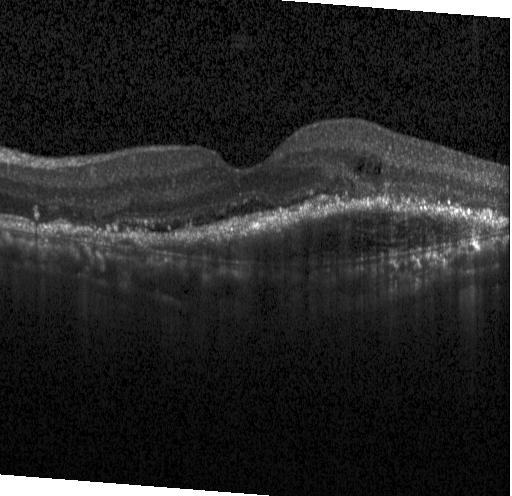 Spectral-domain optical coherence tomography. OCT B-scan — Impression: a choroidal neovascular membrane.